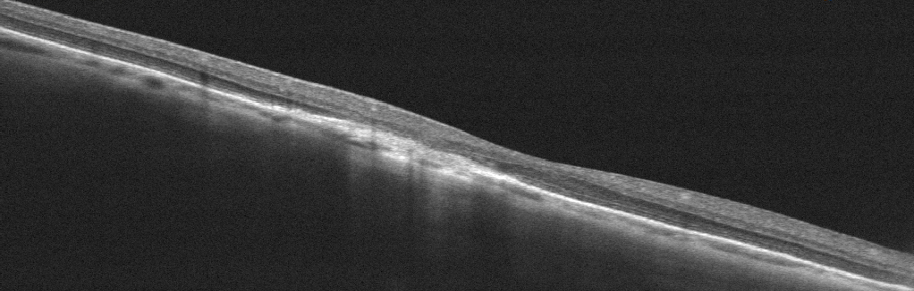
Macular scan; retinal OCT cross-section — The scan shows AMD.